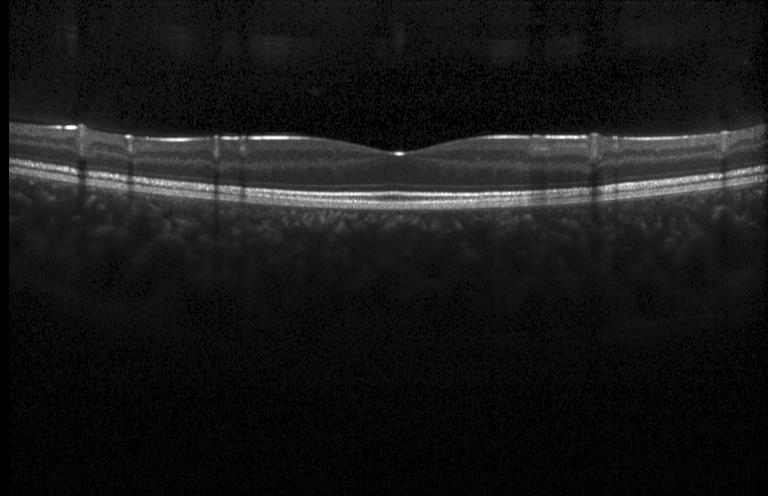

OCT B-scan showing neither choroidal neovascularization, diabetic macular edema, nor drusen.